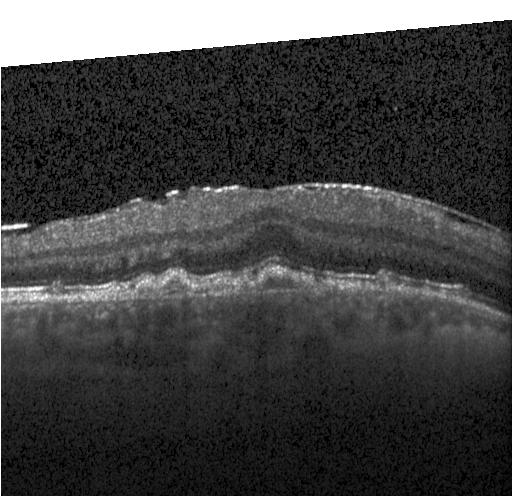

OCT B-scan. Dx: CNV.